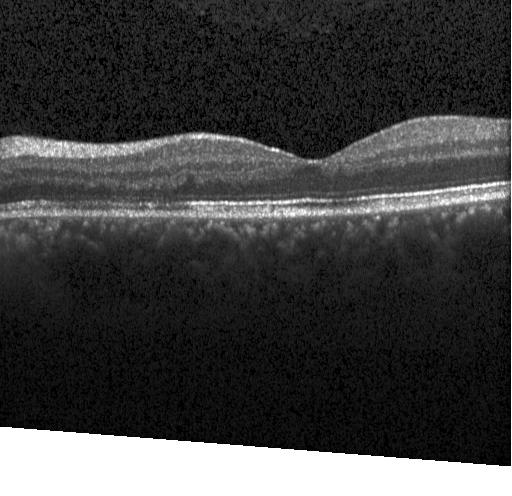 OCT B-scan.
Macular OCT: no evidence of choroidal neovascularization, diabetic macular edema, or drusen.